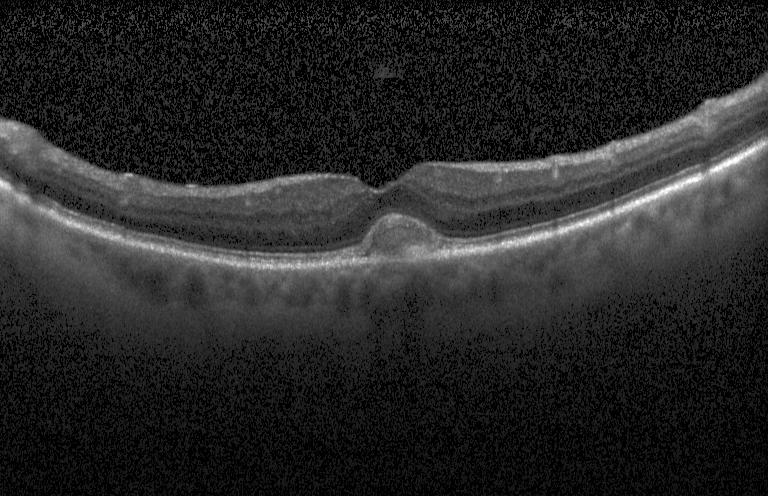

Heidelberg Spectralis OCT system · OCT B-scan — This B-scan demonstrates a choroidal neovascular membrane.